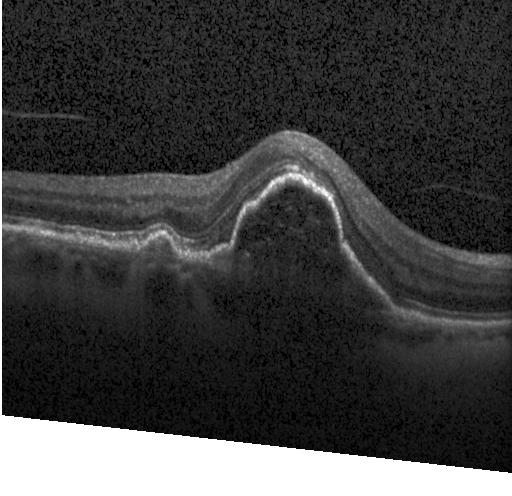

Retinal OCT cross-section.
The scan shows a choroidal neovascular membrane.